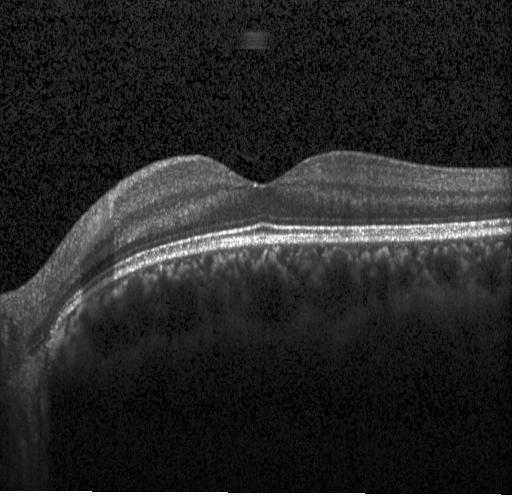
Optical coherence tomography scan. OCT finding: no evidence of CNV, DME, or drusen.